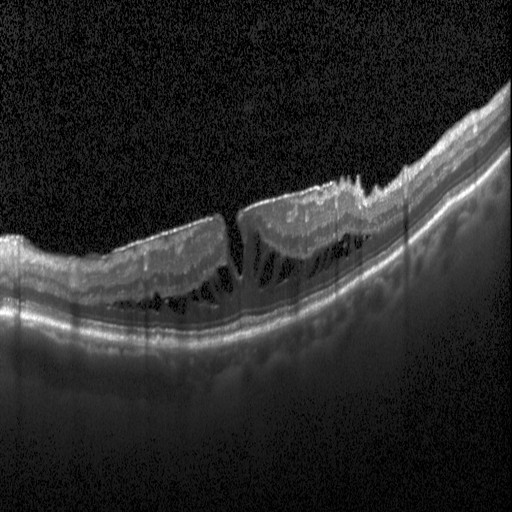 Impression: DME.